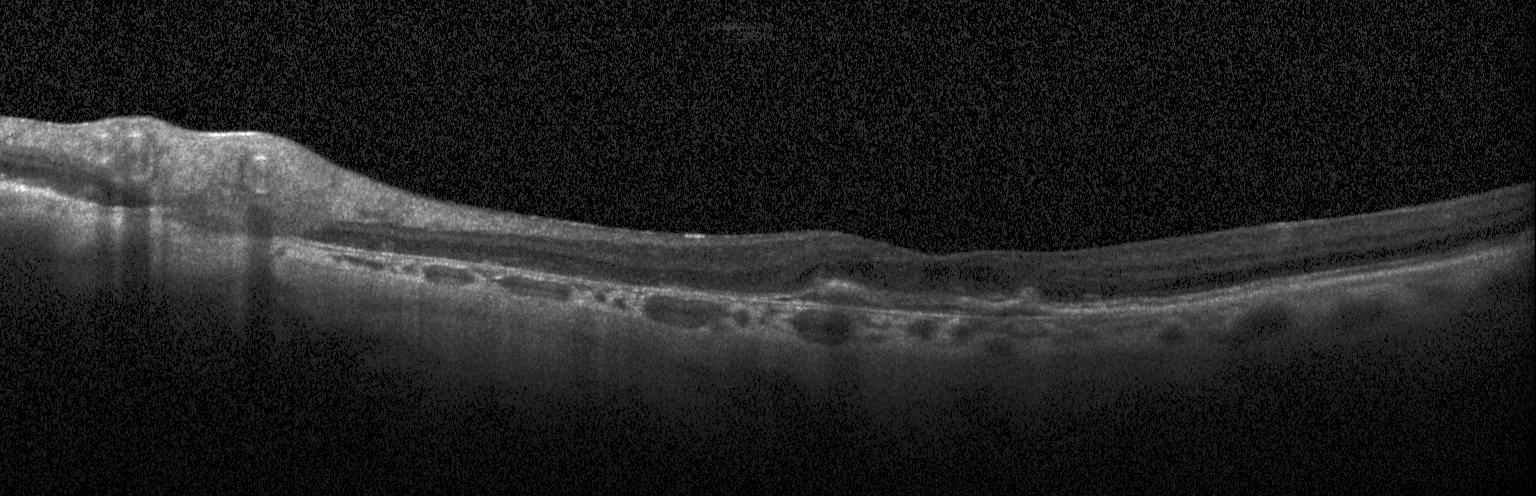

Impression: a choroidal neovascular membrane.